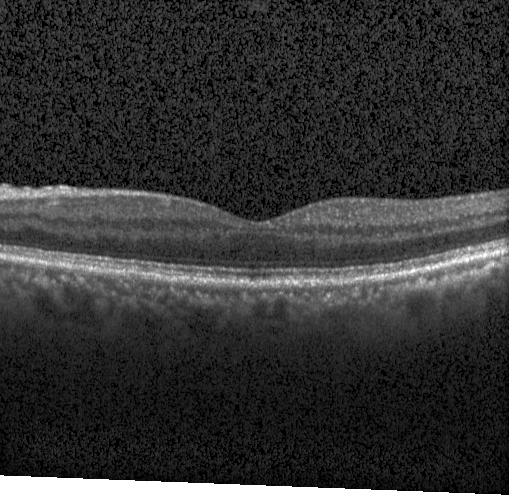 Dx: no choroidal neovascularization, no diabetic macular edema, and no drusen.